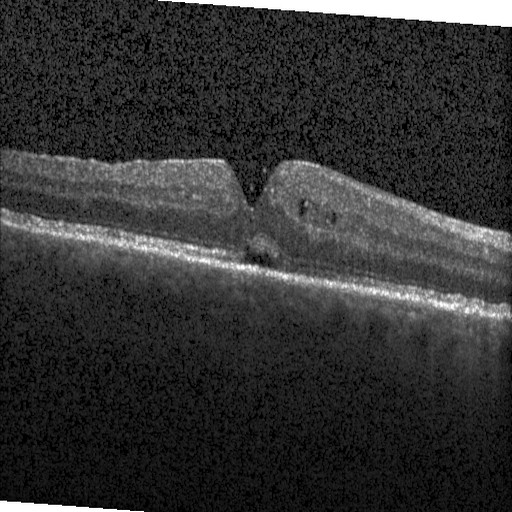
Impression: diabetic macular edema.